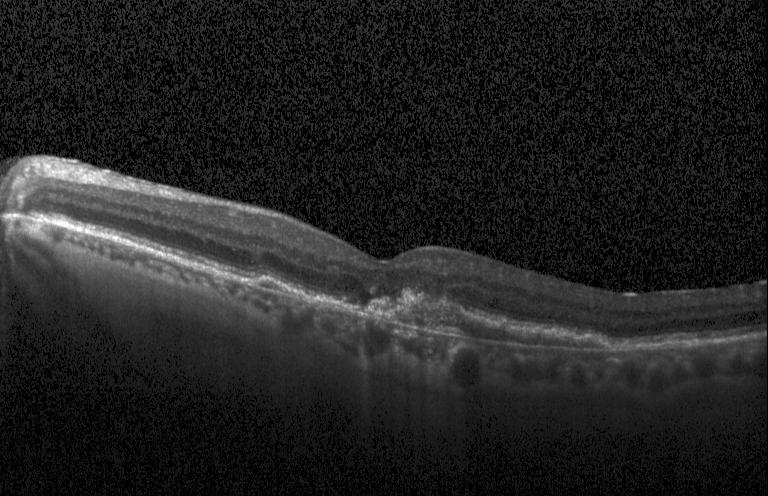

Spectral-domain OCT. OCT B-scan. Dx: a choroidal neovascular membrane.